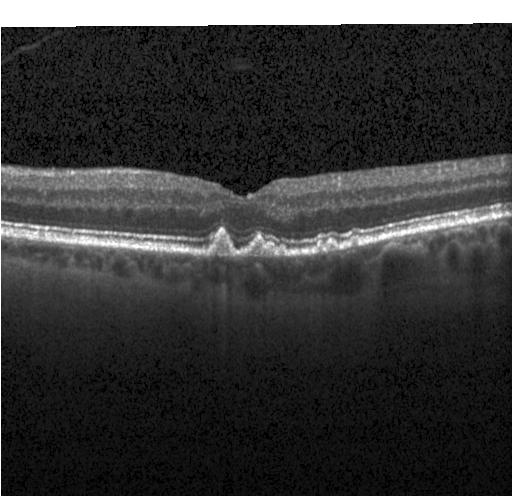

Spectral-domain optical coherence tomography, OCT line scan. This B-scan demonstrates sub-RPE drusenoid deposits.